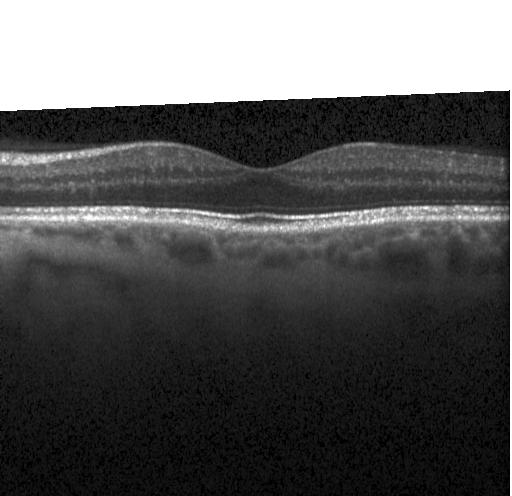
No evidence of choroidal neovascularization, diabetic macular edema, or drusen.